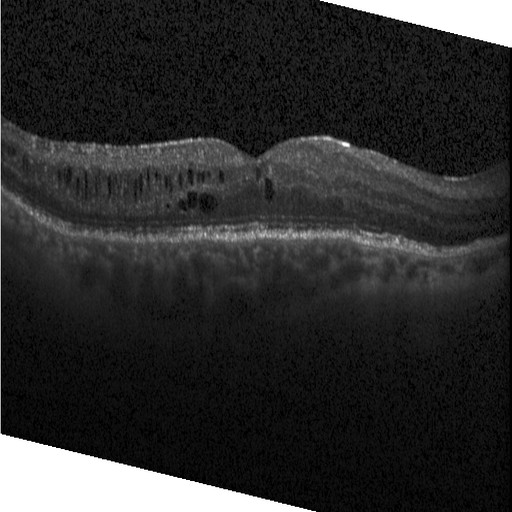 Retinal OCT cross-section · spectral-domain OCT
Diagnosis: DME.